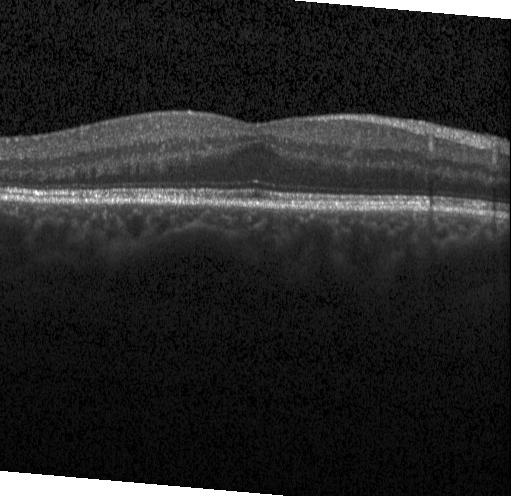

OCT line scan; acquired on a Heidelberg Spectralis.
The scan shows no CNV, DME, or drusen.